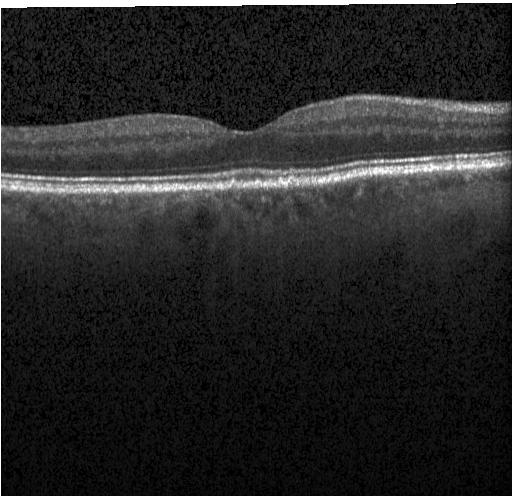

Retinal OCT cross-section. Spectral-domain optical coherence tomography. Heidelberg Spectralis.
This B-scan demonstrates no CNV, DME, or drusen.